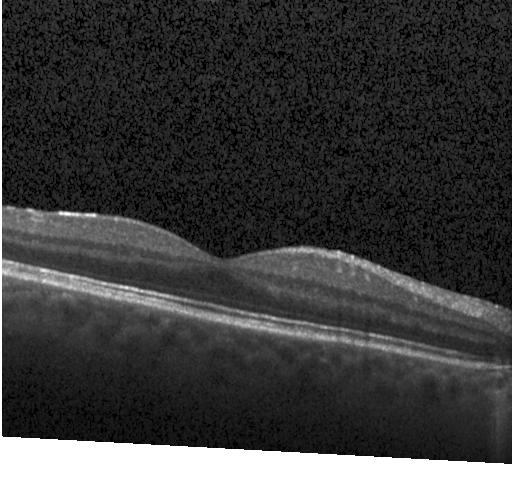

Retinal OCT cross-section · acquired on a Heidelberg Spectralis · spectral-domain OCT · through the macula. The scan shows neither choroidal neovascularization, diabetic macular edema, nor drusen.